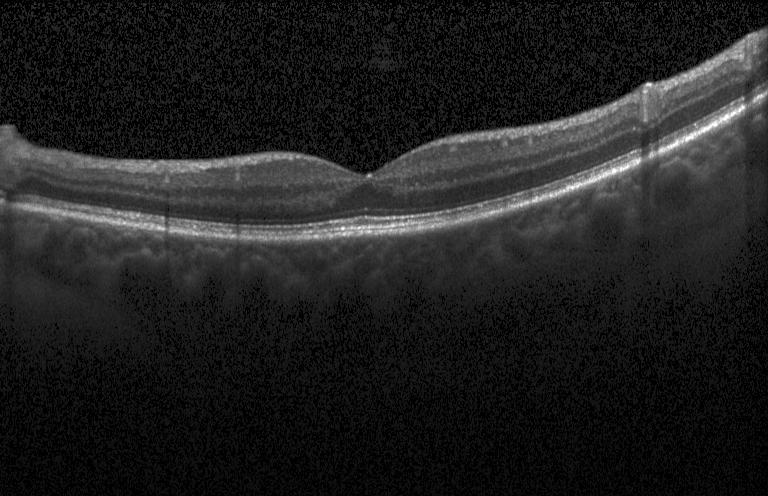 OCT line scan — Finding: no evidence of choroidal neovascularization, diabetic macular edema, or drusen.